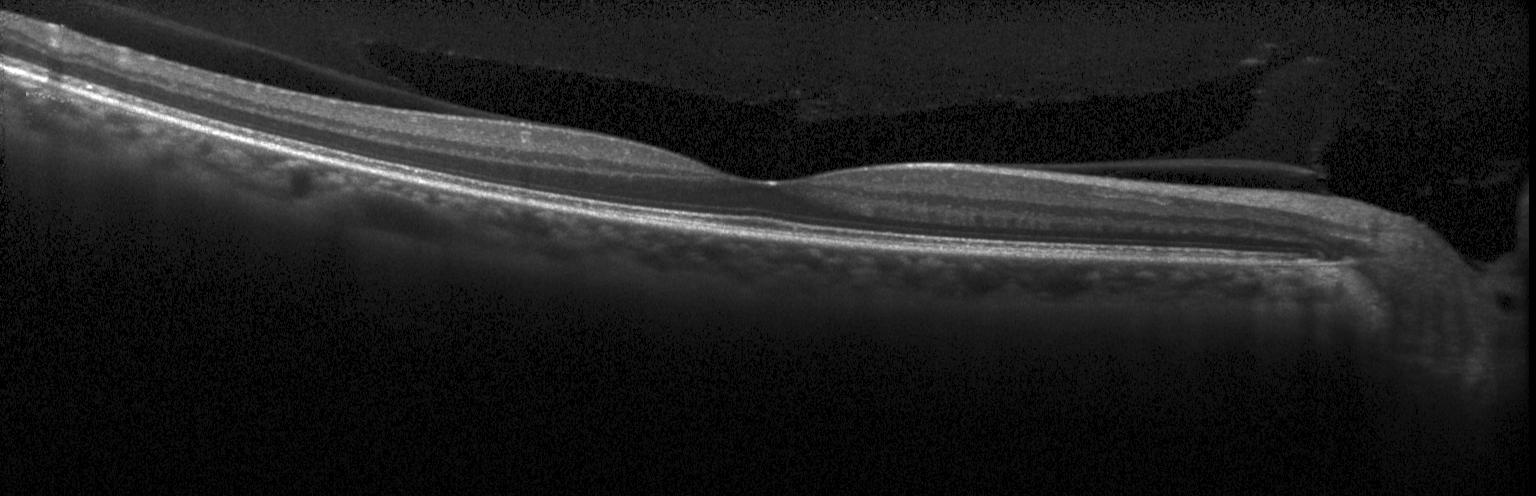
OCT finding: no CNV, no DME, and no drusen.